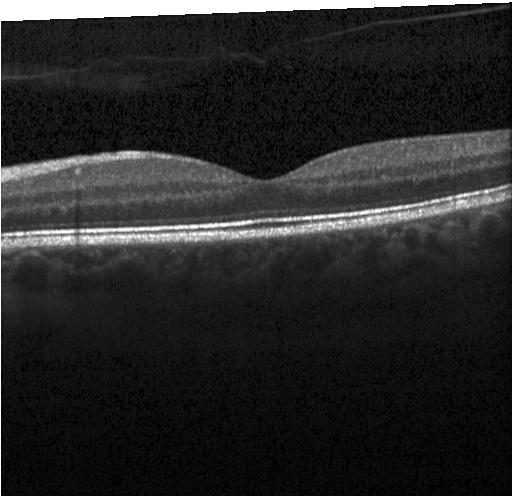
Finding: no choroidal neovascularization, no diabetic macular edema, and no drusen.